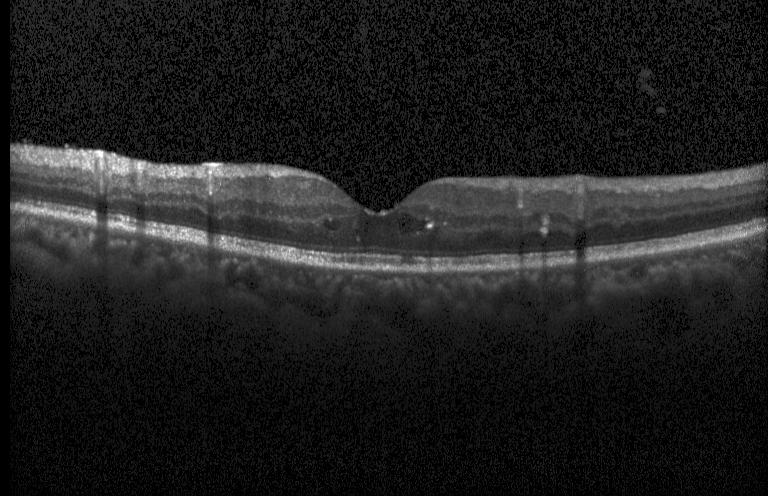 OCT B-scan; instrument: Heidelberg Spectralis; centered on the fovea; SD-OCT. Impression: diabetic macular edema (DME).